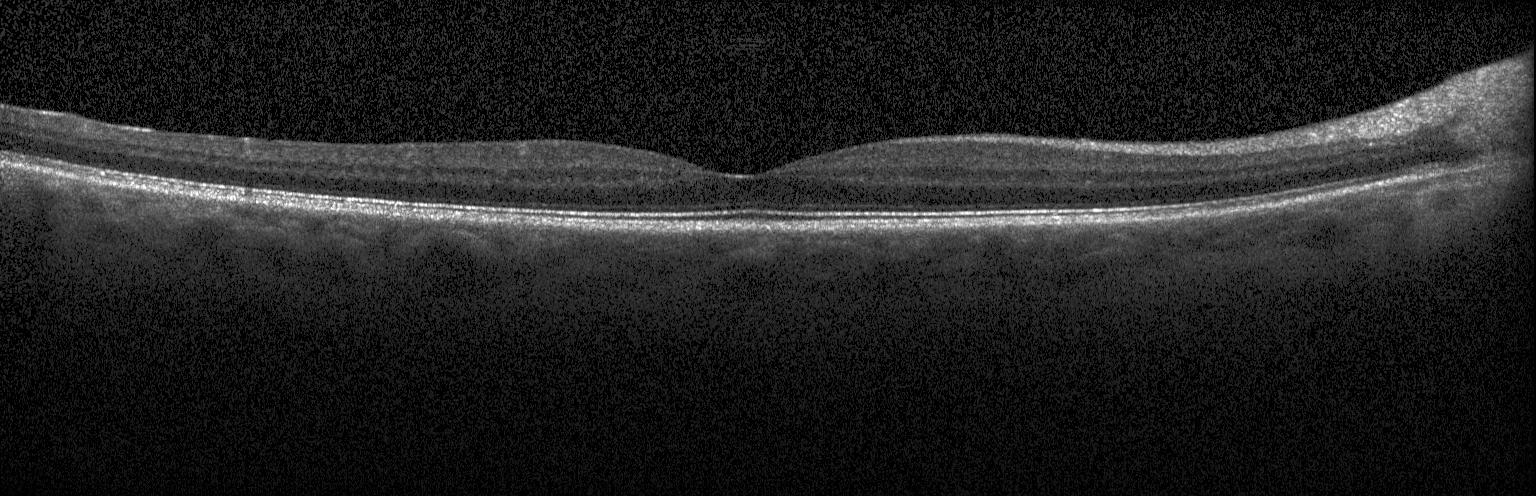
The scan shows no choroidal neovascularization, no diabetic macular edema, and no drusen.